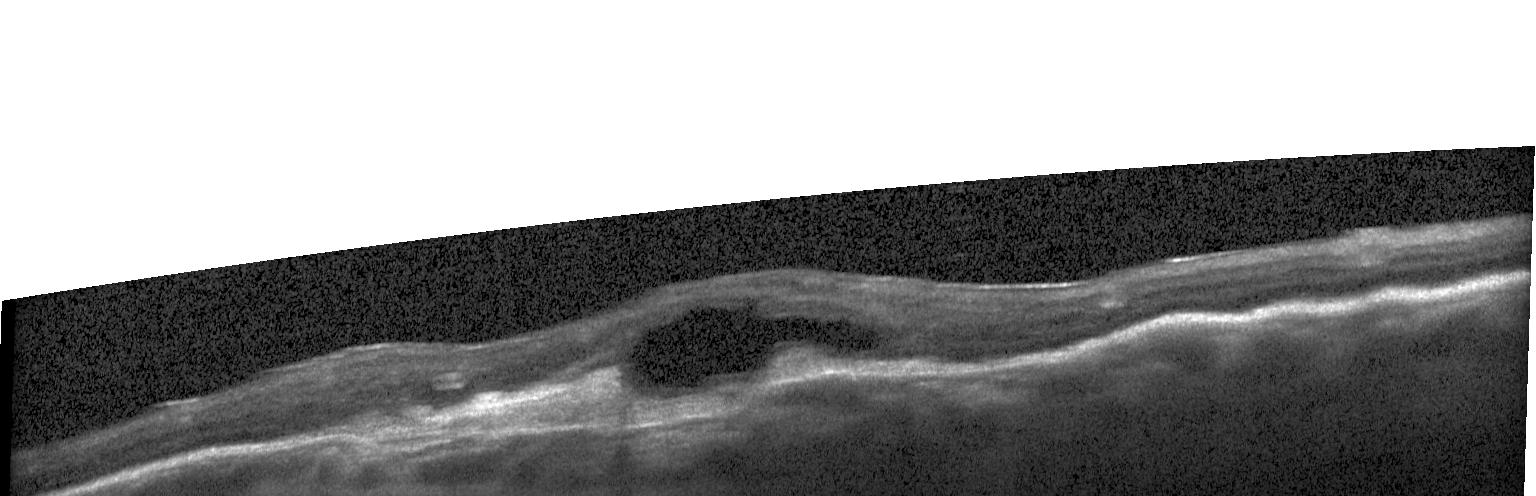
Retinal OCT B-scan
Dx: choroidal neovascularization (CNV).